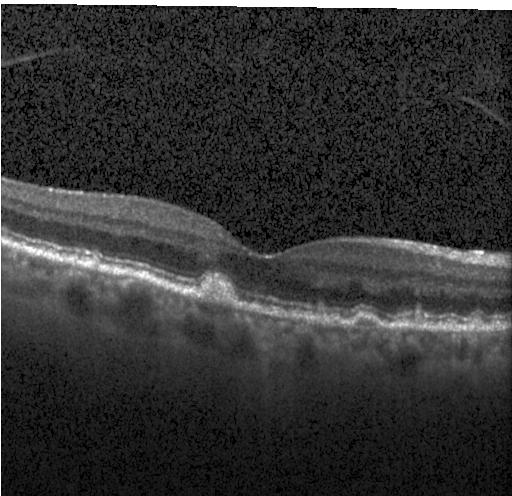
Impression: multiple drusen.